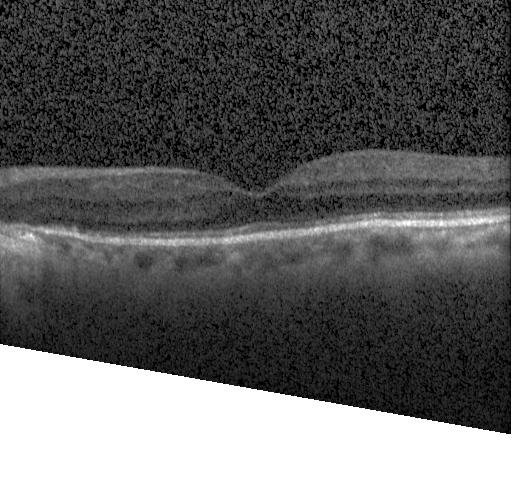
Retinal OCT cross-section, instrument: Heidelberg Spectralis.
Assessment: no choroidal neovascularization, diabetic macular edema, or drusen.